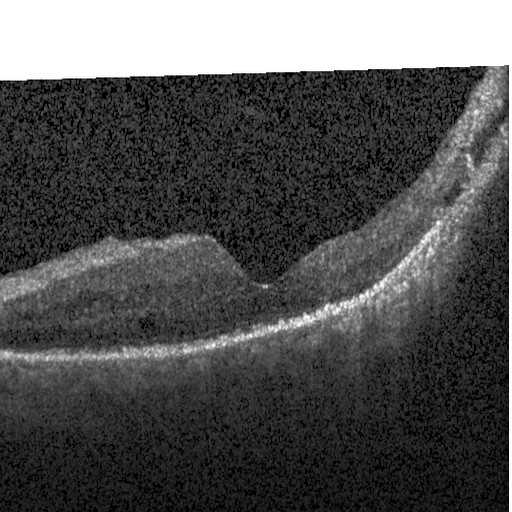 Assessment: diabetic macular edema (DME).